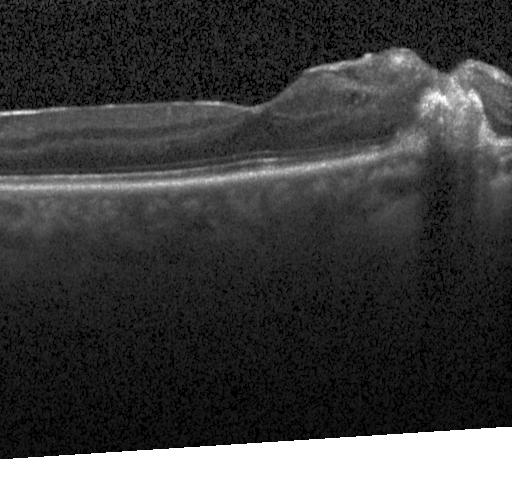

Spectral-domain OCT B-scan: CNV.